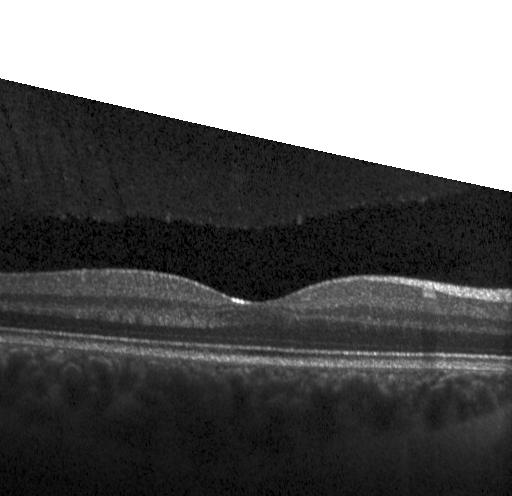
Spectral-domain OCT; OCT B-scan; centered on the fovea. Dx: neither choroidal neovascularization, diabetic macular edema, nor drusen.